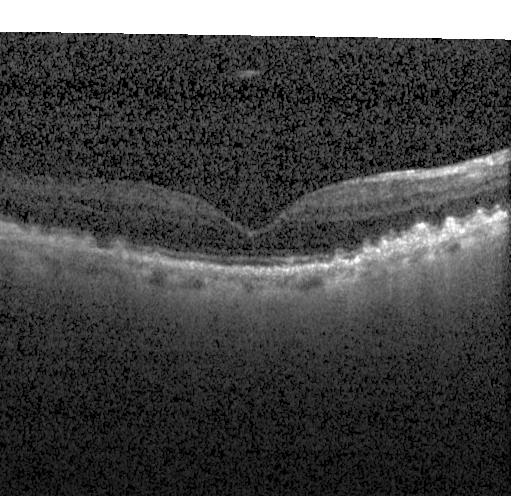

Macular OCT demonstrating sub-RPE drusenoid deposits.